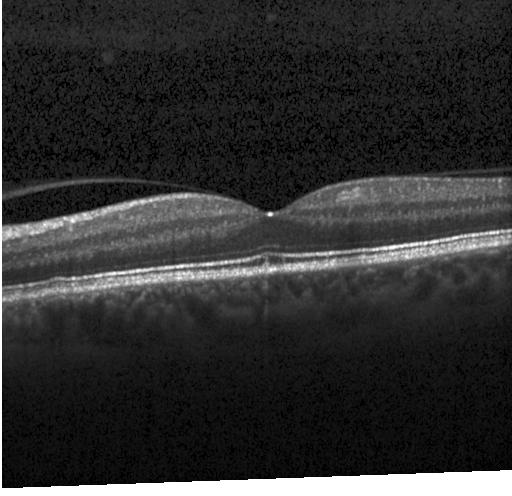

OCT B-scan showing neither CNV, DME, nor drusen.